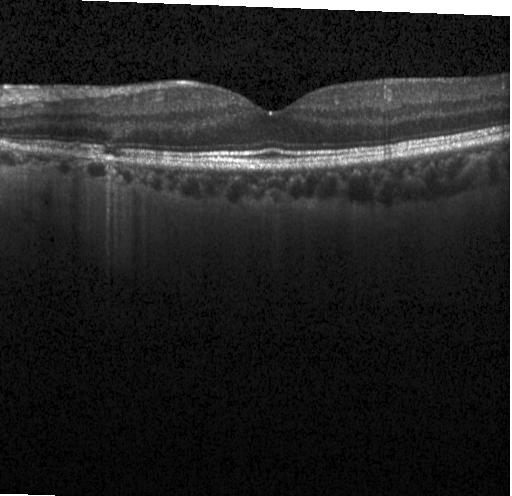

Optical coherence tomography scan; spectral-domain optical coherence tomography; fovea-centered; acquired on a Heidelberg Spectralis
The scan shows no choroidal neovascularization, diabetic macular edema, or drusen.